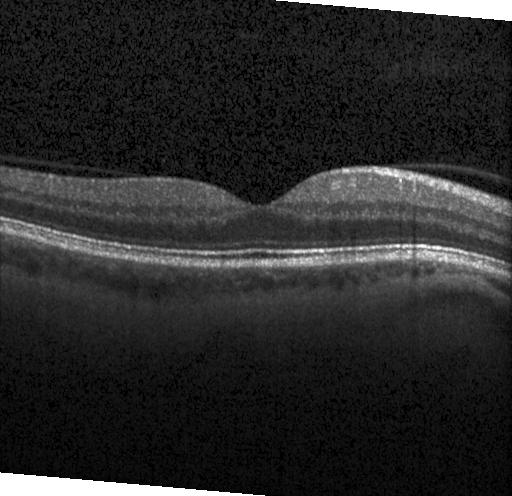

OCT B-scan showing no CNV, DME, or drusen.